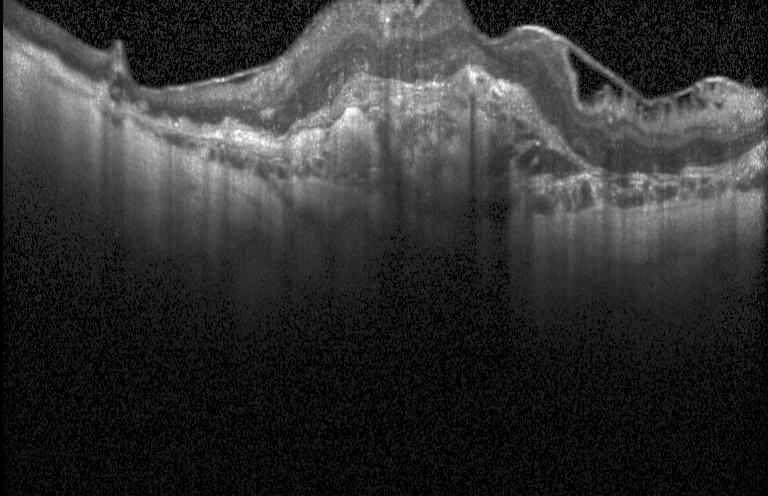 Acquired on a Heidelberg Spectralis, SD-OCT, OCT line scan — This B-scan demonstrates CNV.